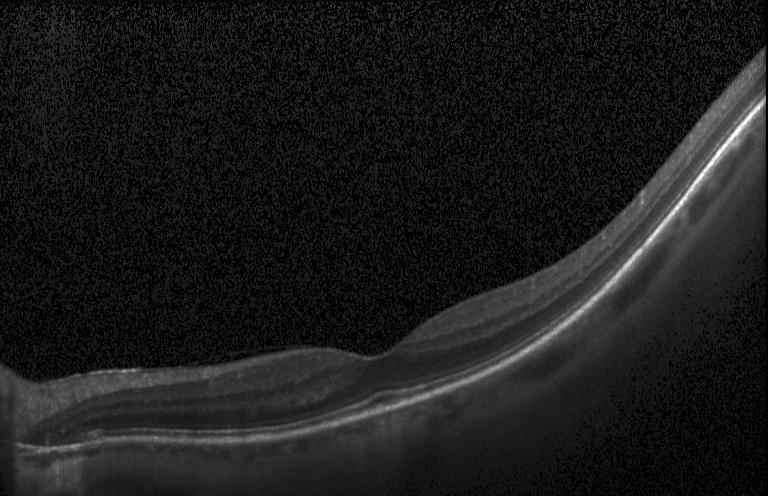

Retinal OCT cross-section
Neither choroidal neovascularization, diabetic macular edema, nor drusen.